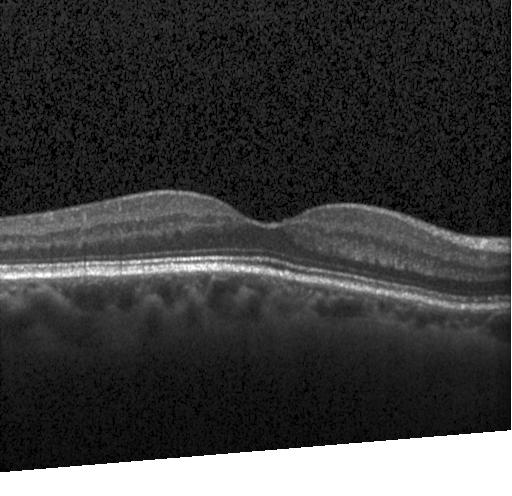 Macular OCT demonstrating no choroidal neovascularization, diabetic macular edema, or drusen.